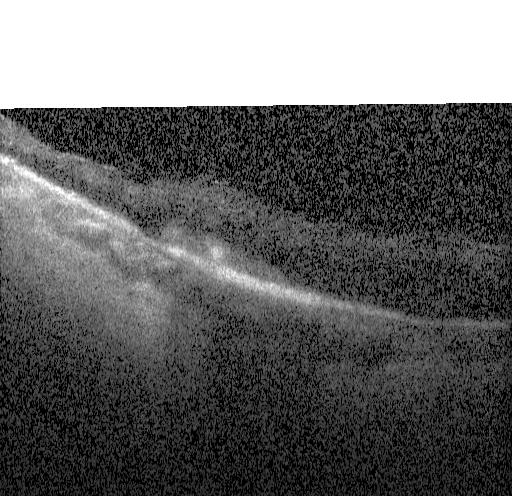 OCT B-scan; spectral-domain optical coherence tomography
A choroidal neovascular membrane.